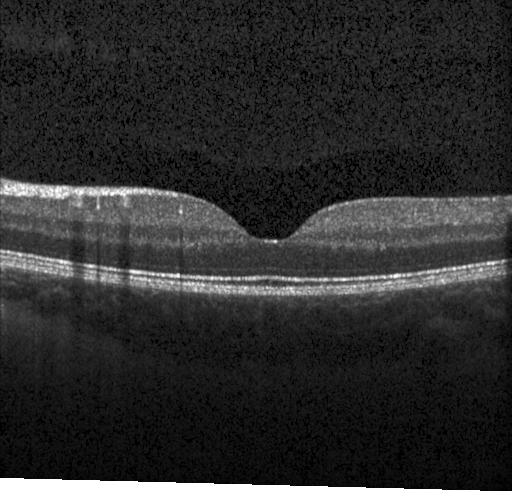 OCT B-scan
Finding: no CNV, no DME, and no drusen.